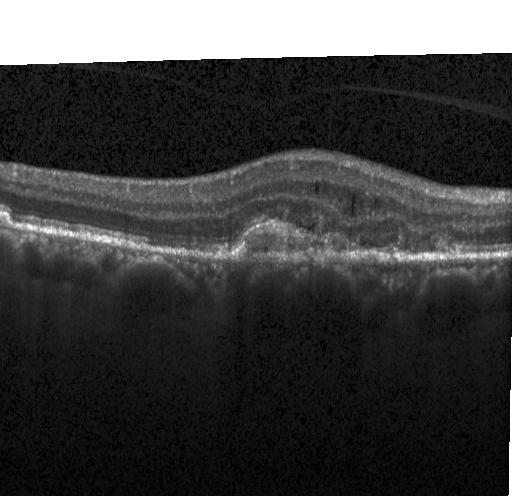

Heidelberg Spectralis OCT system; OCT line scan. Dx: CNV.